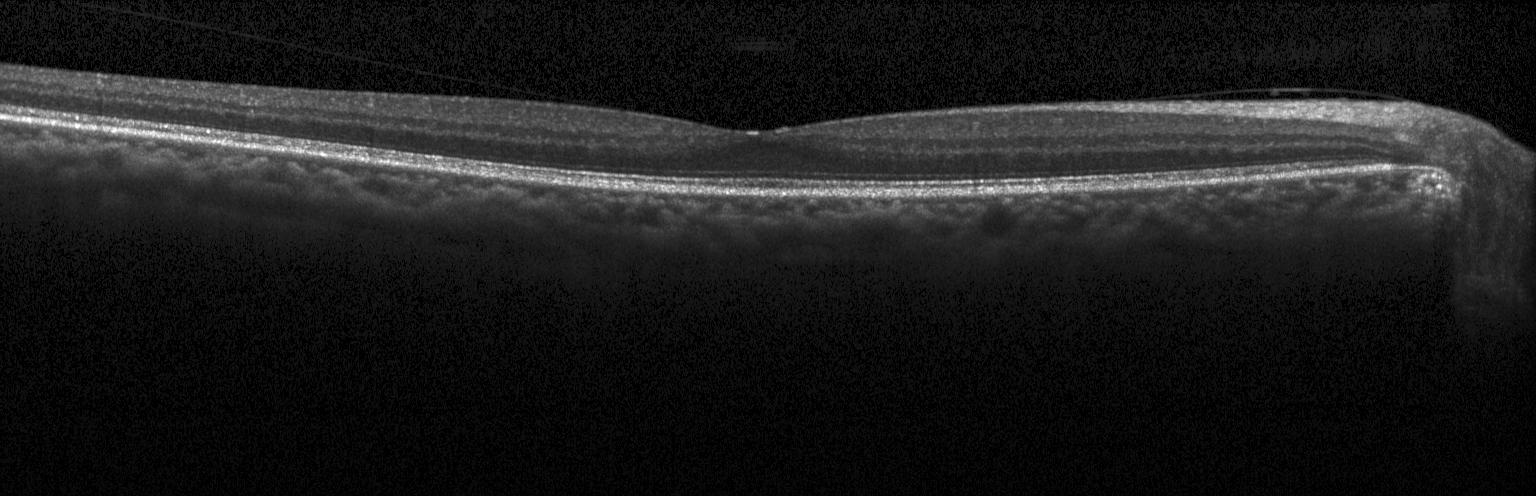

Diagnosis: no choroidal neovascularization, no diabetic macular edema, and no drusen.